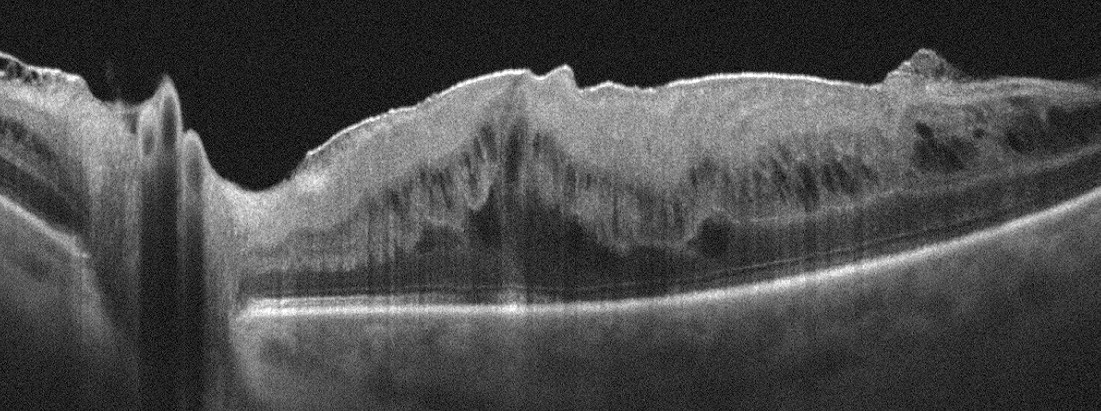
OCT scan showing ERM.